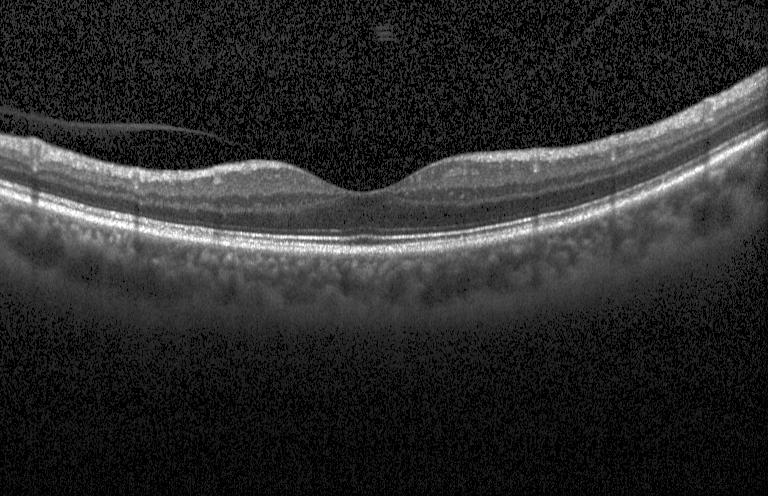

Diagnosis: no choroidal neovascularization, diabetic macular edema, or drusen.